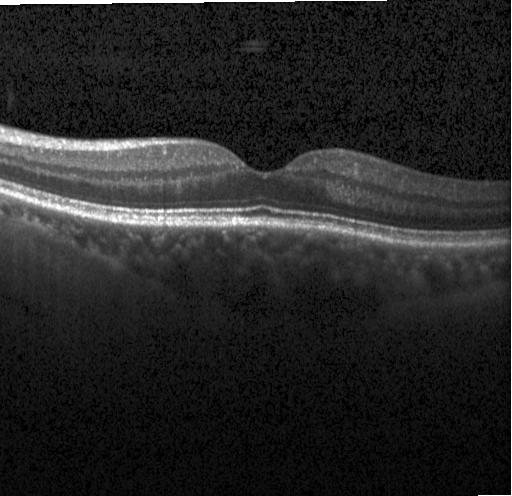 Heidelberg Spectralis OCT system; retinal OCT cross-section; centered on the fovea. Impression: neither CNV, DME, nor drusen.